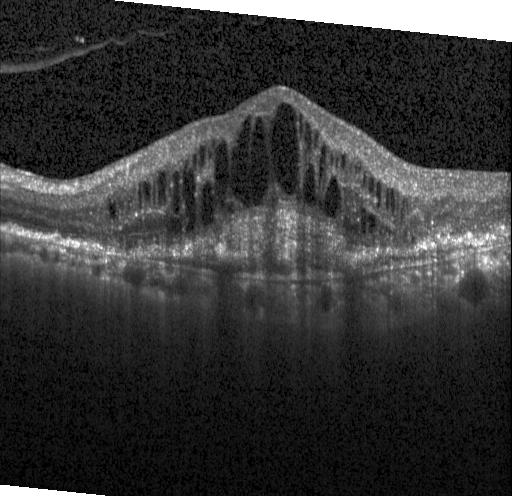
Optical coherence tomography B-scan — Finding: choroidal neovascularization.